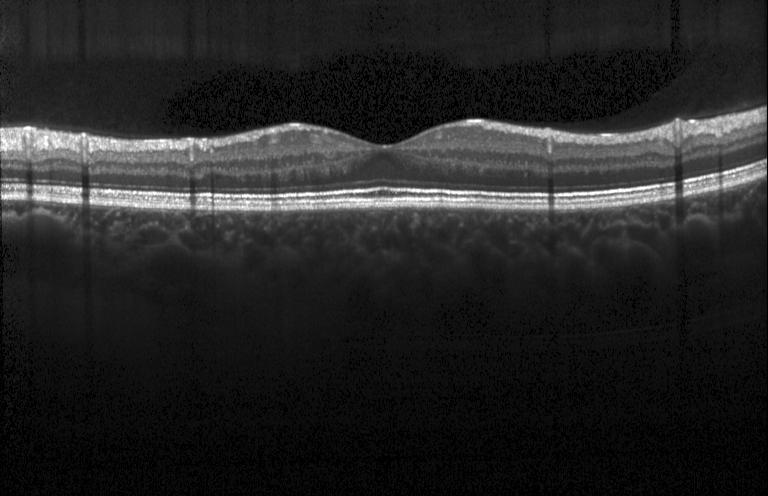
OCT B-scan. The scan shows no evidence of choroidal neovascularization, diabetic macular edema, or drusen.